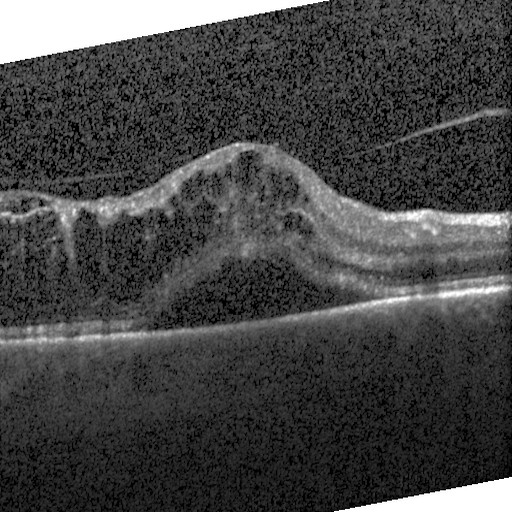 Horizontal scan through the fovea; OCT line scan.
Finding: diabetic macular edema.